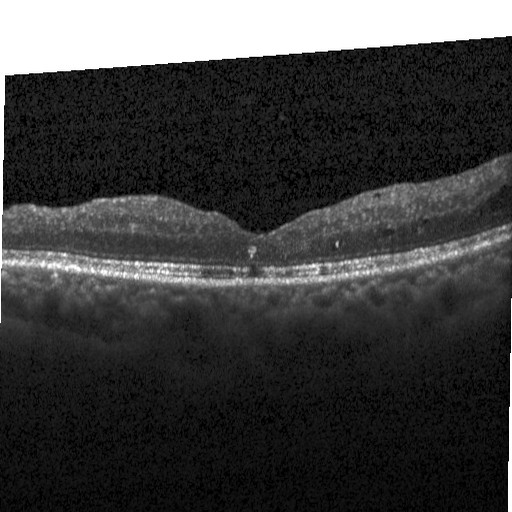 Finding: diabetic macular edema.